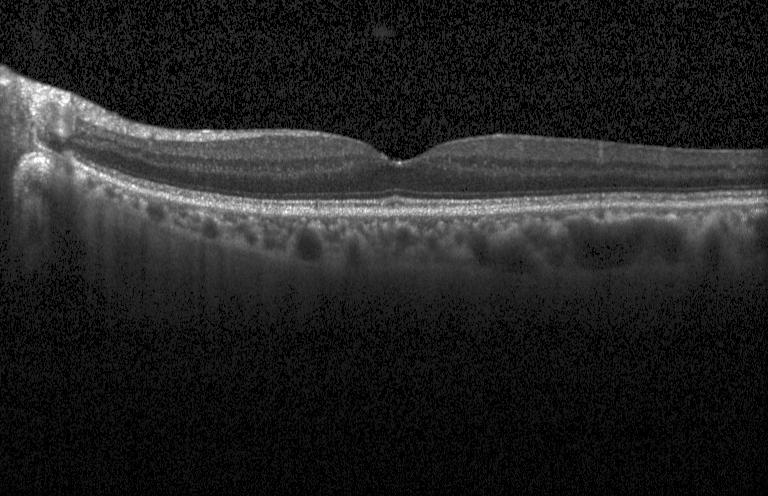 Spectral-domain OCT · retinal OCT cross-section · acquired on a Heidelberg Spectralis · horizontal scan through the fovea — Impression: no choroidal neovascularization, diabetic macular edema, or drusen.